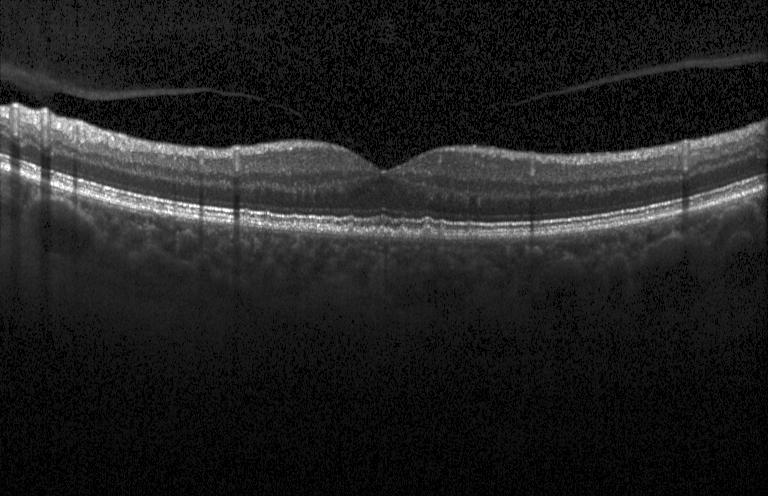
Retinal OCT B-scan · acquired on a Heidelberg Spectralis · SD-OCT — Finding: multiple drusen.